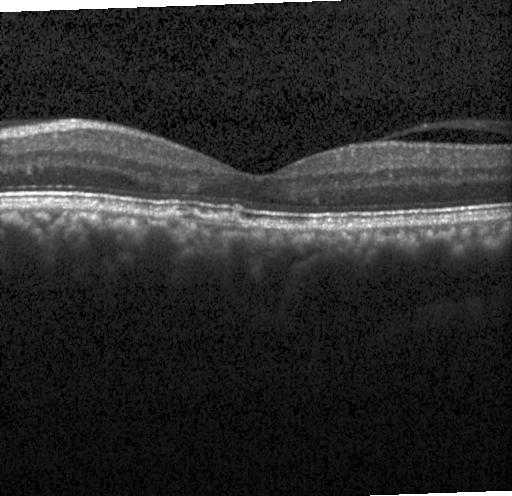 Optical coherence tomography B-scan — Diagnosis: multiple drusen.